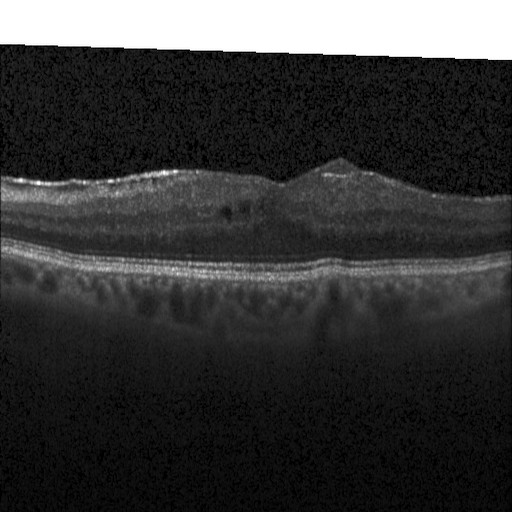 Heidelberg Spectralis OCT system, optical coherence tomography B-scan
Impression: diabetic macular edema.